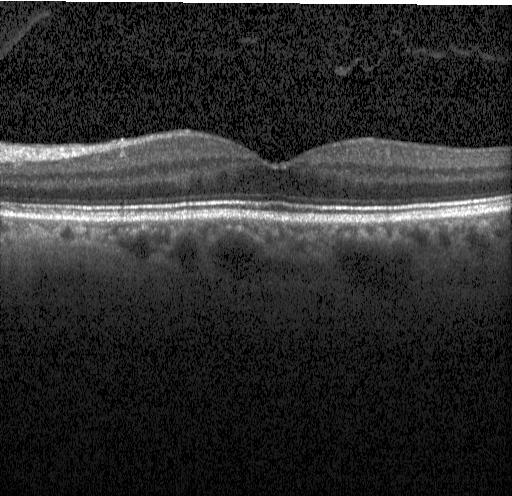

Spectral-domain OCT, OCT B-scan, fovea-centered. Assessment: no choroidal neovascularization, no diabetic macular edema, and no drusen.